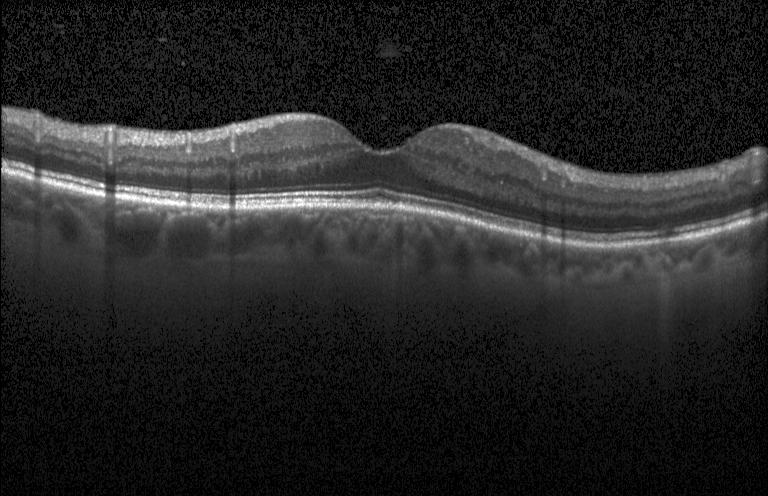
Spectral-domain OCT. Retinal OCT B-scan. Acquired on a Heidelberg Spectralis
Diagnosis: no evidence of CNV, DME, or drusen.